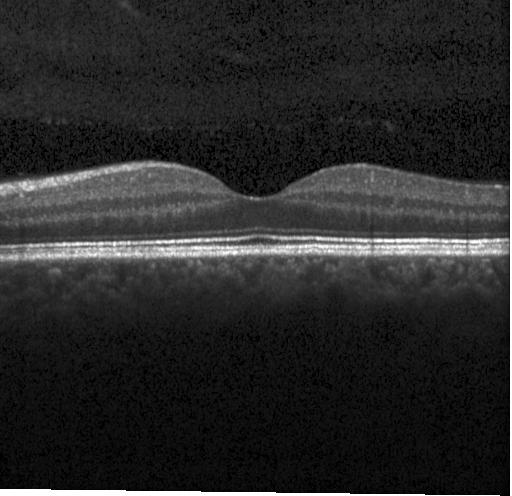 Retinal OCT cross-section. OCT finding: no CNV, DME, or drusen.